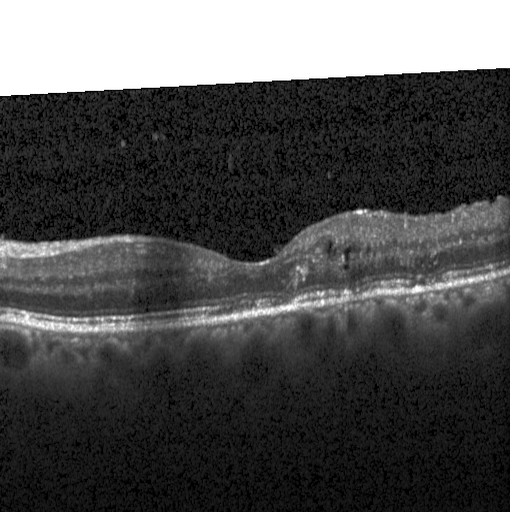

OCT B-scan; SD-OCT; centered on the fovea
OCT finding: diabetic macular edema.